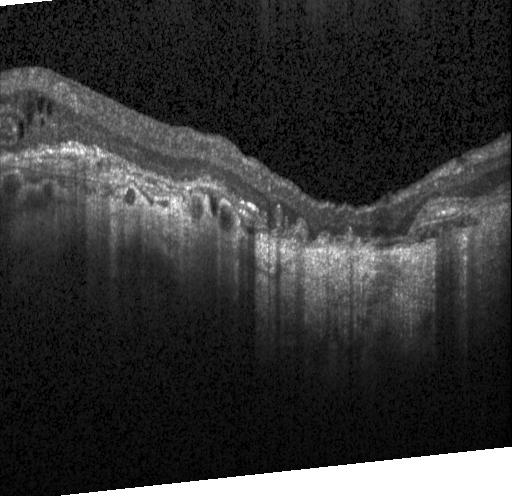 Assessment: a choroidal neovascular membrane.